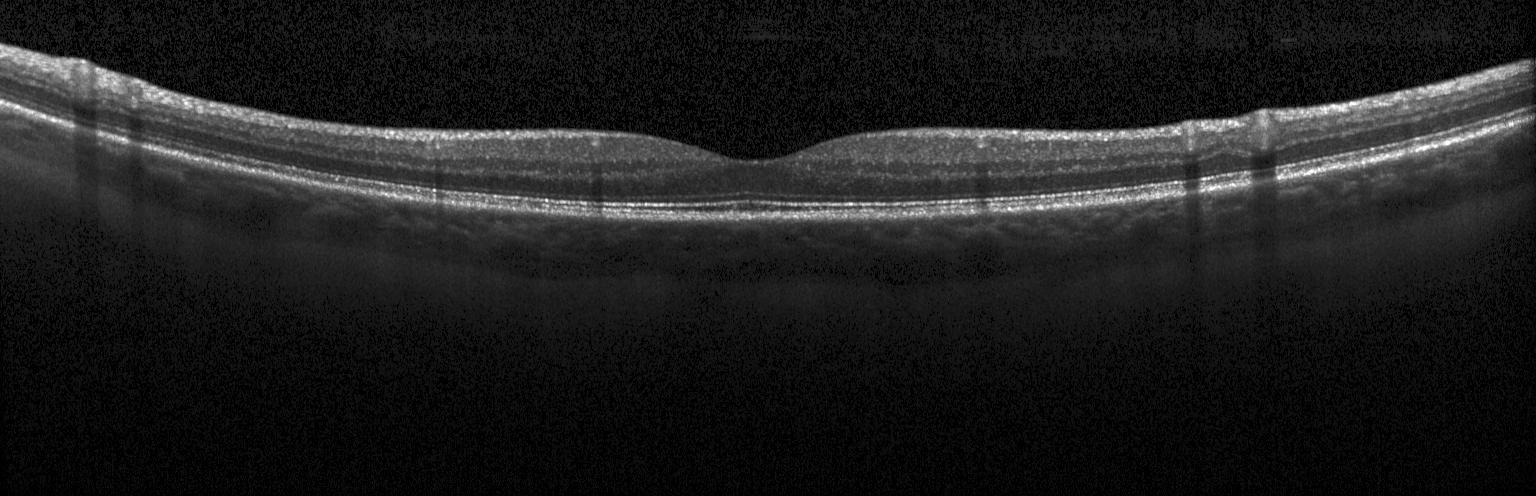

Retinal OCT cross-section.
Dx: no choroidal neovascularization, no diabetic macular edema, and no drusen.